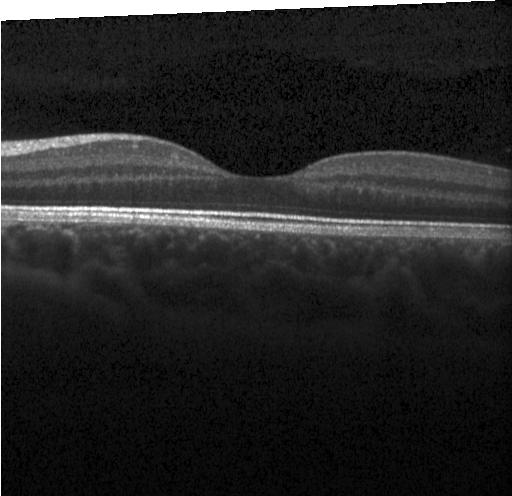

Retinal OCT cross-section · Heidelberg Spectralis OCT system · centered on the fovea. Macular OCT: neither choroidal neovascularization, diabetic macular edema, nor drusen.